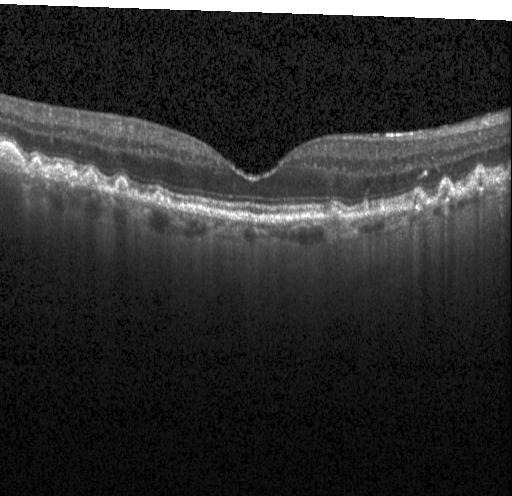
Spectral-domain optical coherence tomography; OCT line scan; instrument: Heidelberg Spectralis
This B-scan demonstrates multiple drusen.